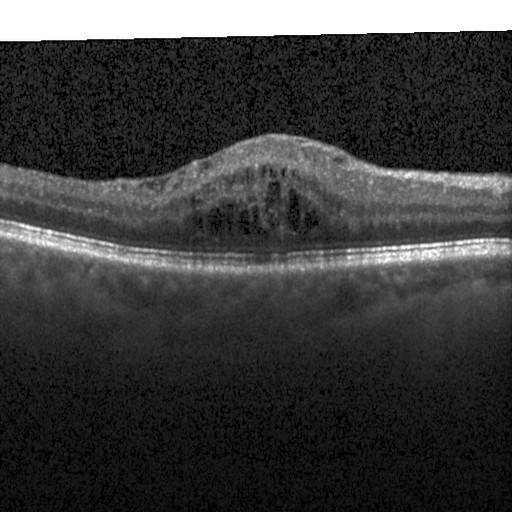

OCT scan showing diabetic macular edema.